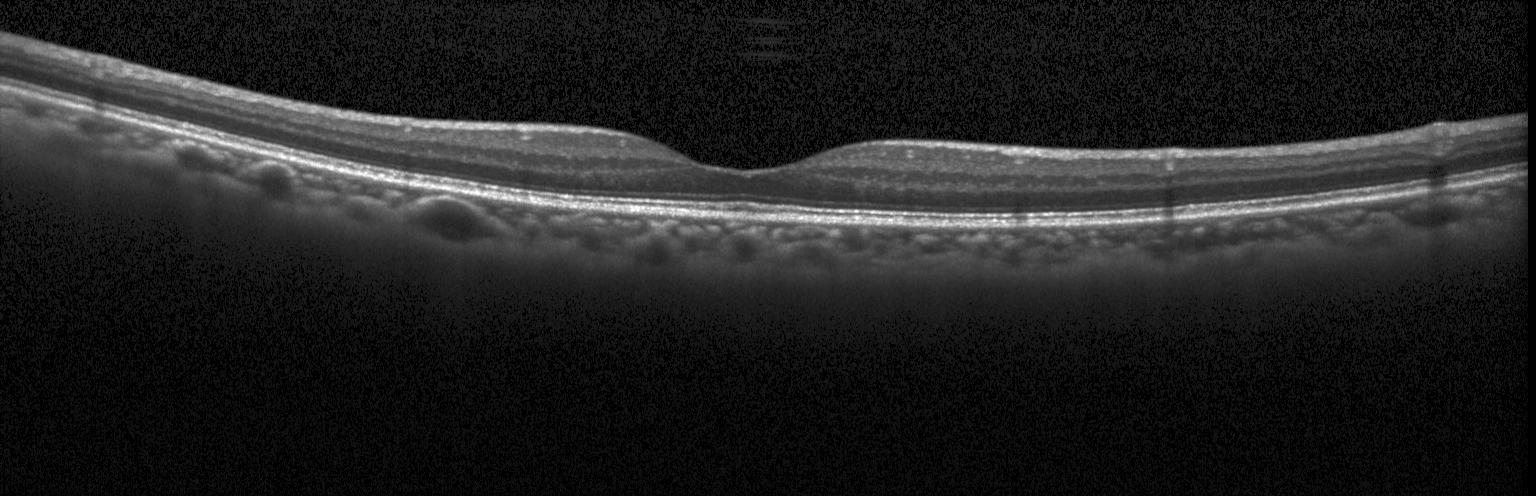

SD-OCT; fovea-centered; optical coherence tomography B-scan
Finding: no evidence of choroidal neovascularization, diabetic macular edema, or drusen.